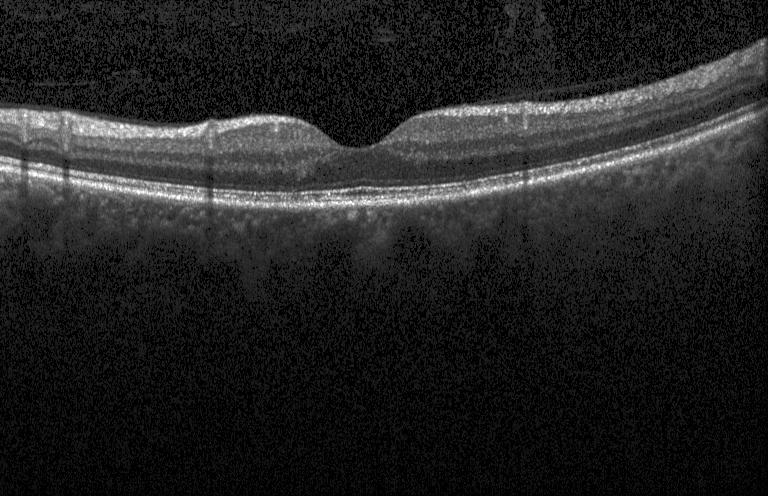
OCT B-scan showing neither choroidal neovascularization, diabetic macular edema, nor drusen.